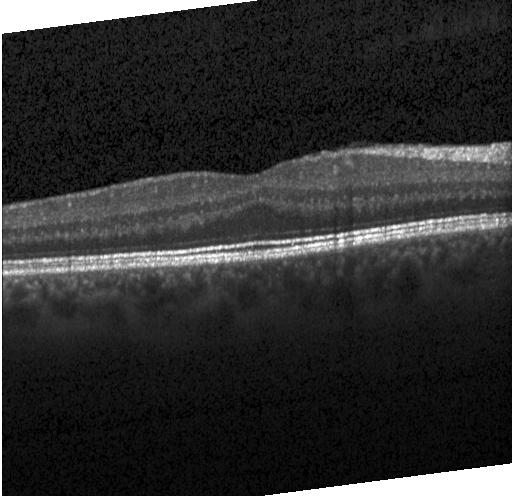 Heidelberg Spectralis; retinal OCT cross-section — Finding: no evidence of choroidal neovascularization, diabetic macular edema, or drusen.